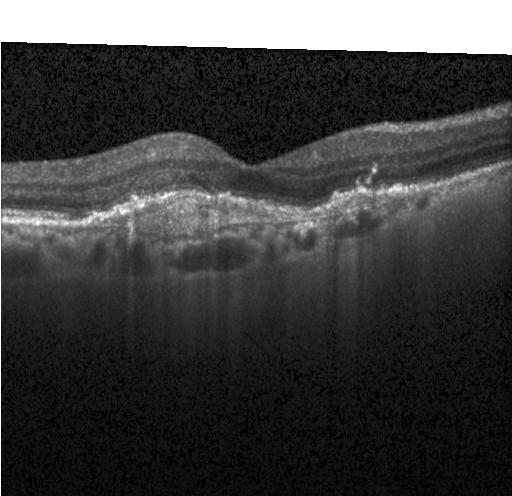
Retinal OCT B-scan, horizontal scan through the fovea, SD-OCT
Diagnosis: a choroidal neovascular membrane.